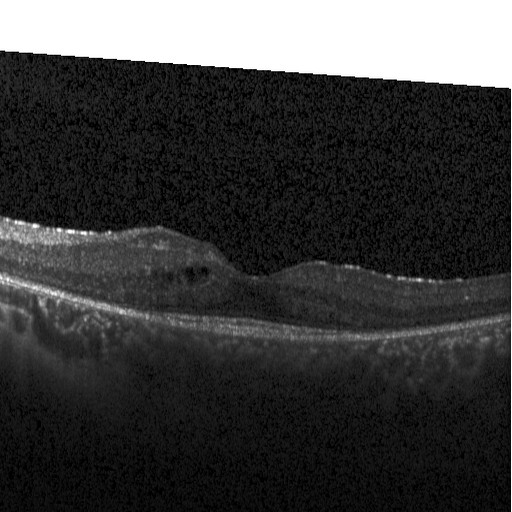 Instrument: Heidelberg Spectralis · spectral-domain optical coherence tomography · optical coherence tomography B-scan · centered on the fovea.
Macular OCT: diabetic macular edema.